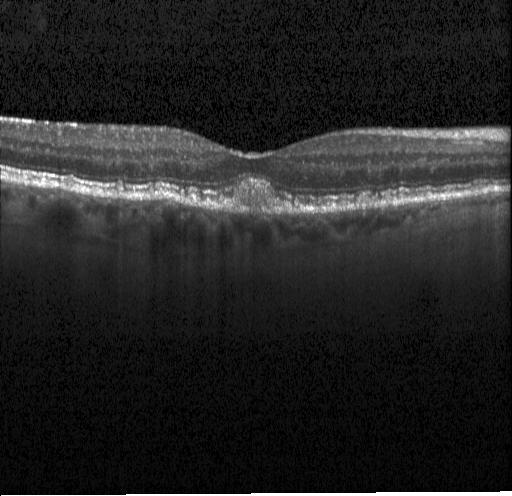 Retinal OCT cross-section.
Assessment: sub-RPE drusenoid deposits.